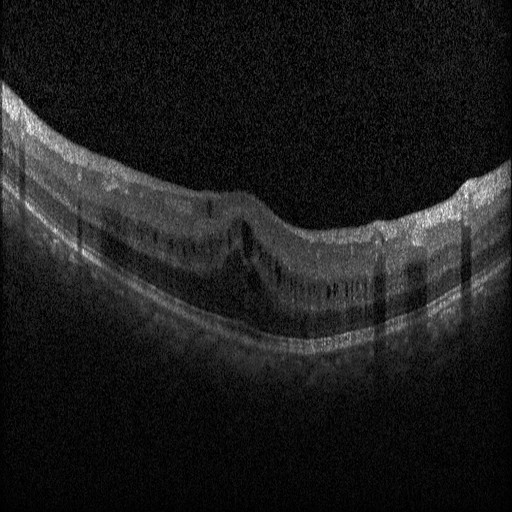
OCT line scan. The scan shows diabetic macular edema.